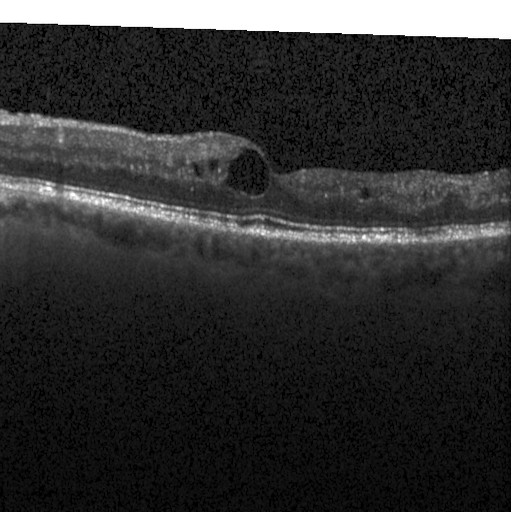 Macular scan. Optical coherence tomography B-scan. Acquired on a Heidelberg Spectralis — Diagnosis: diabetic macular edema.